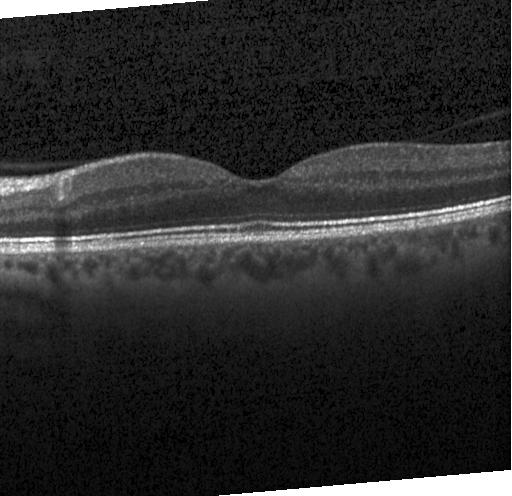
Retinal OCT cross-section; Heidelberg Spectralis OCT system; centered on the fovea; spectral-domain OCT — Impression: no choroidal neovascularization, diabetic macular edema, or drusen.